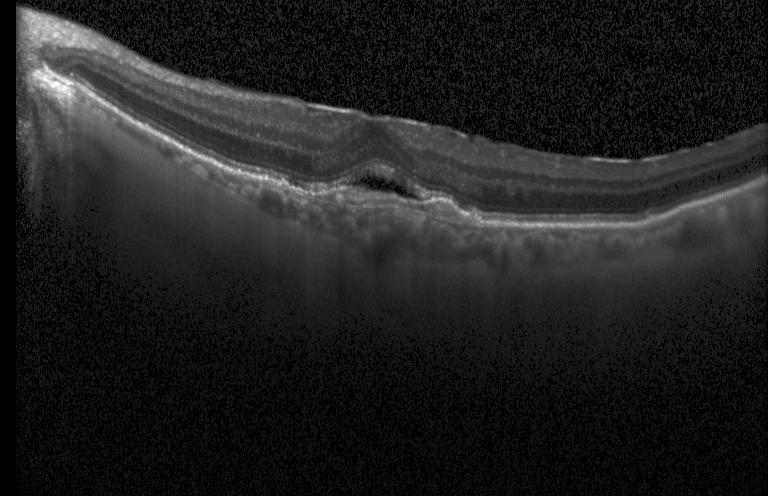

Impression: a choroidal neovascular membrane.